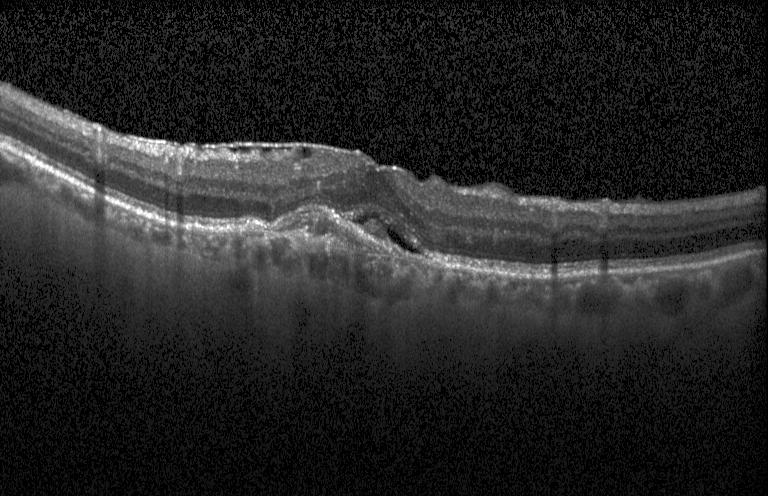

Retinal OCT cross-section — Impression: CNV.